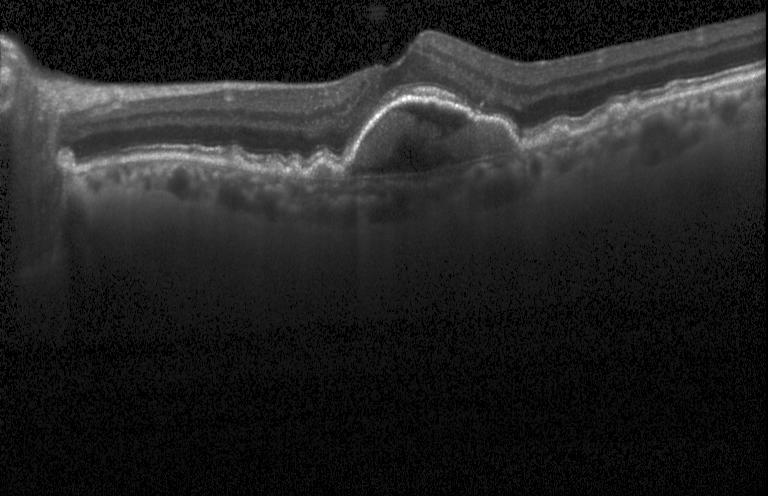

SD-OCT · centered on the fovea · OCT B-scan · Heidelberg Spectralis OCT system.
OCT finding: sub-RPE drusenoid deposits.